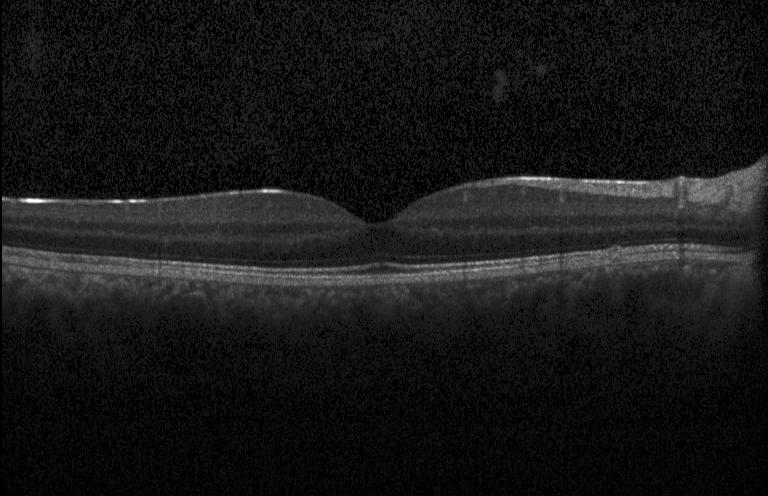 Macular OCT: no choroidal neovascularization, no diabetic macular edema, and no drusen.